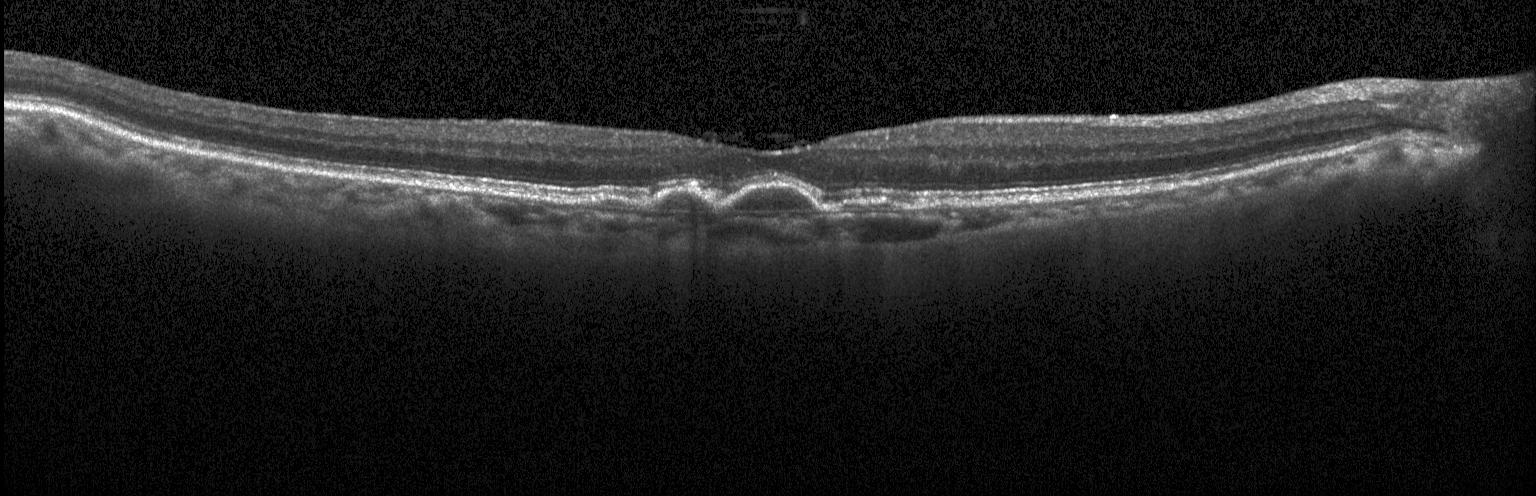

Spectral-domain OCT; optical coherence tomography B-scan; horizontal scan through the fovea.
Dx: a choroidal neovascular membrane.